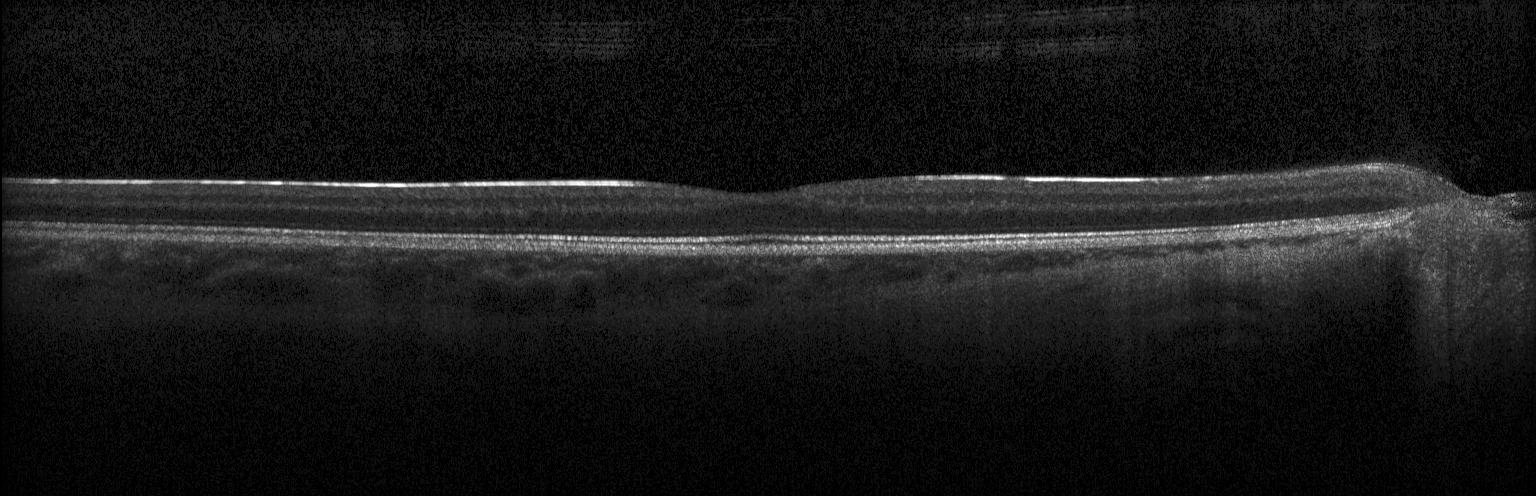

Spectral-domain OCT B-scan: no choroidal neovascularization, diabetic macular edema, or drusen.